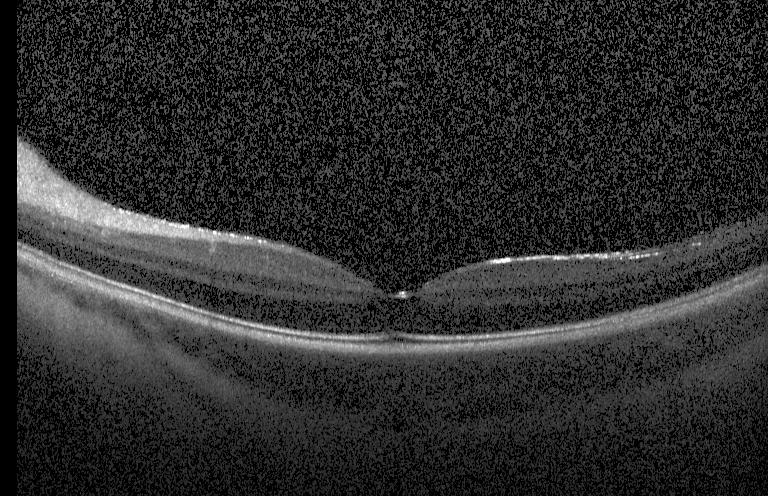 Spectral-domain optical coherence tomography; OCT B-scan — Finding: no evidence of choroidal neovascularization, diabetic macular edema, or drusen.